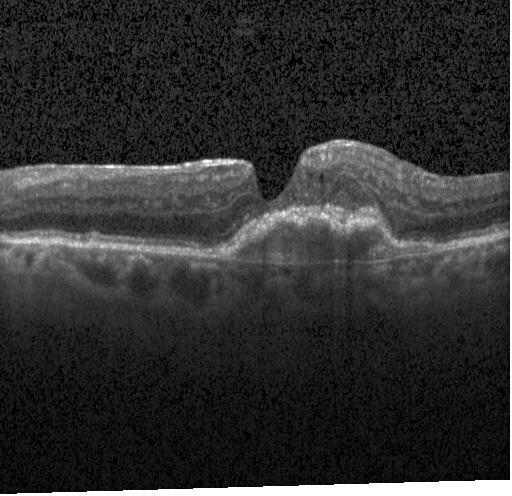

Impression: choroidal neovascularization (CNV).